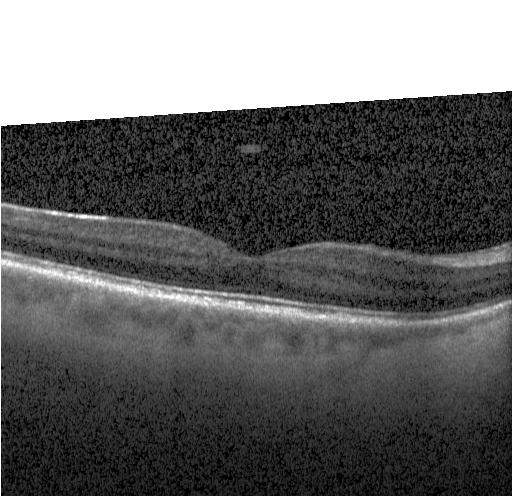 Neither choroidal neovascularization, diabetic macular edema, nor drusen.